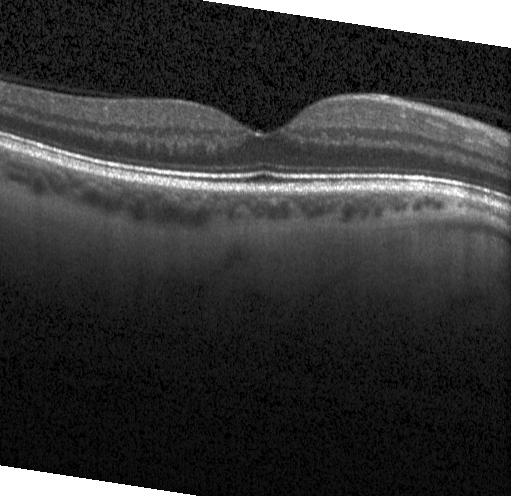 Impression: neither CNV, DME, nor drusen.